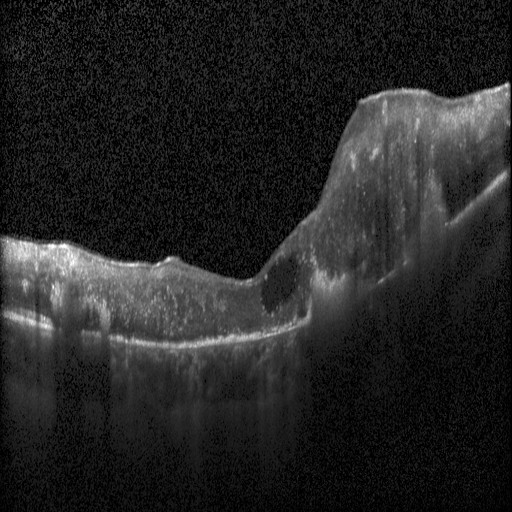

Spectral-domain optical coherence tomography, OCT line scan — This B-scan demonstrates diabetic macular edema.